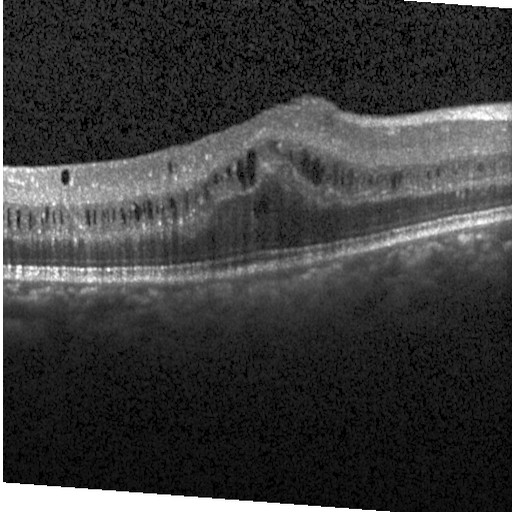 Retinal OCT cross-section · horizontal scan through the fovea · SD-OCT · Heidelberg Spectralis OCT system — Dx: DME.